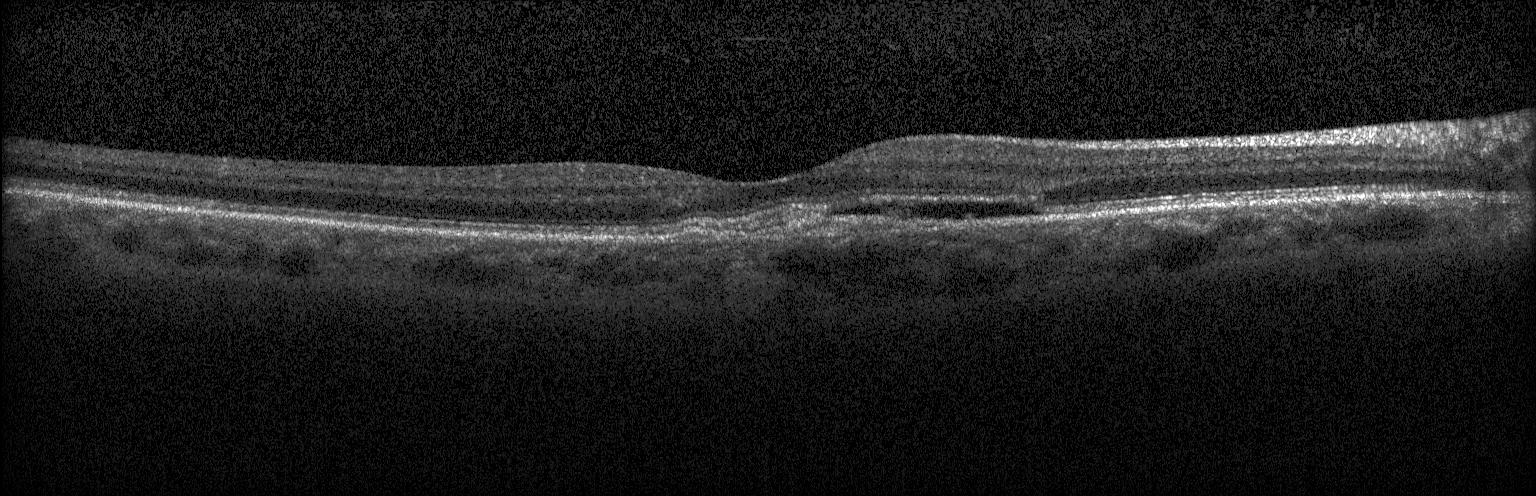

Retinal OCT cross-section
Dx: a choroidal neovascular membrane.